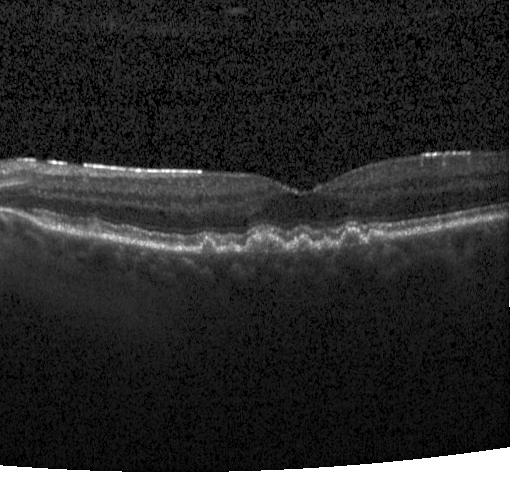
Heidelberg Spectralis; optical coherence tomography scan; SD-OCT; through the macula — Impression: multiple drusen.